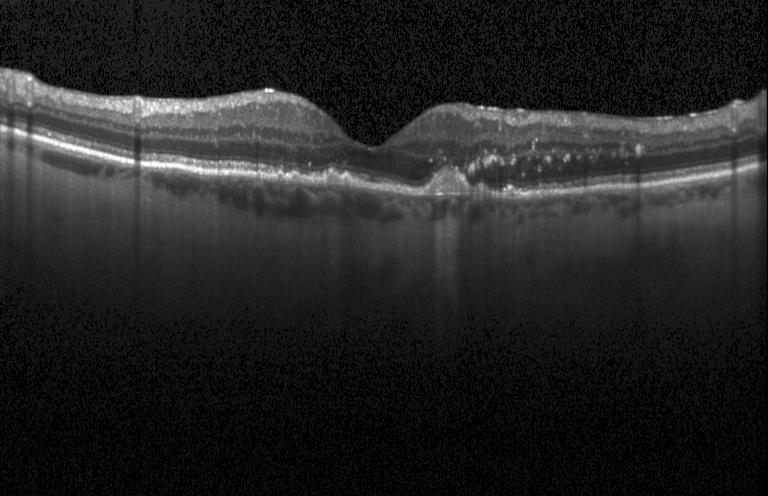
Diagnosis: sub-RPE drusenoid deposits.